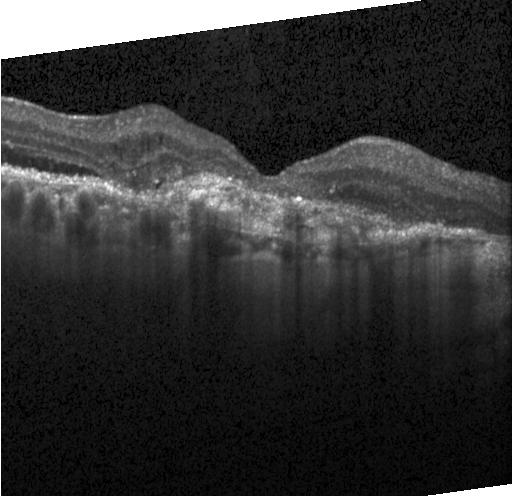
Optical coherence tomography scan — The scan shows a choroidal neovascular membrane.